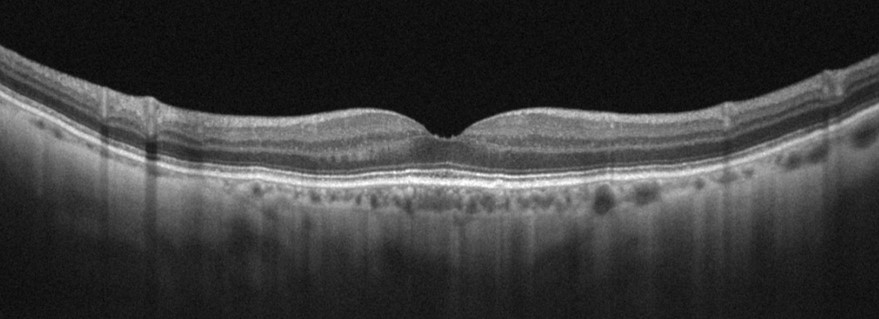 OCT B-scan showing no AMD, DME, ERM, RAO, RVO, or VID.